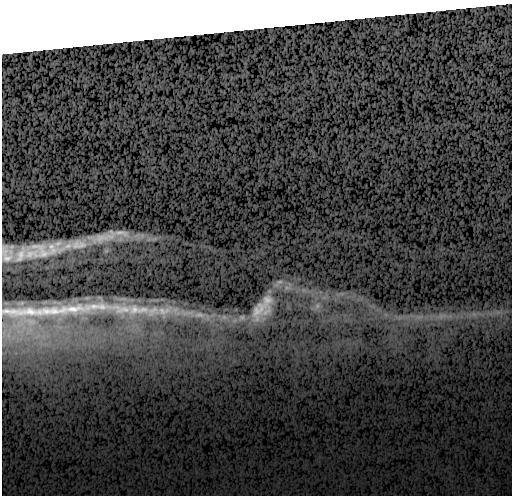
Heidelberg Spectralis. Horizontal scan through the fovea. Spectral-domain OCT. Retinal OCT cross-section — Diagnosis: CNV.